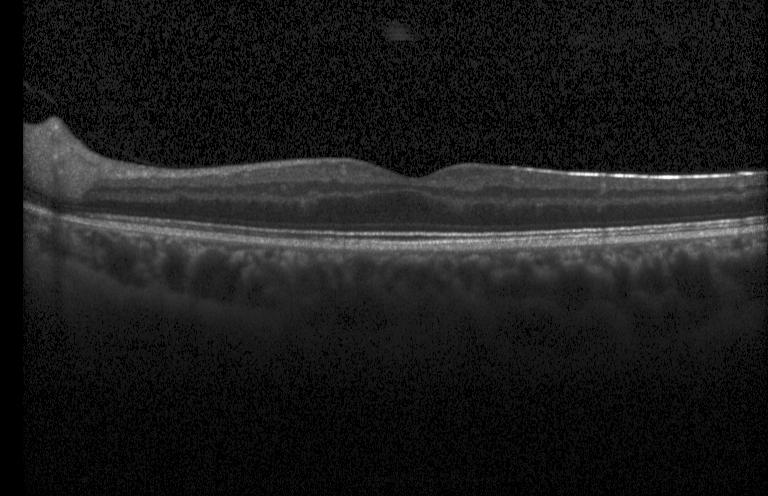

This B-scan demonstrates no choroidal neovascularization, diabetic macular edema, or drusen.